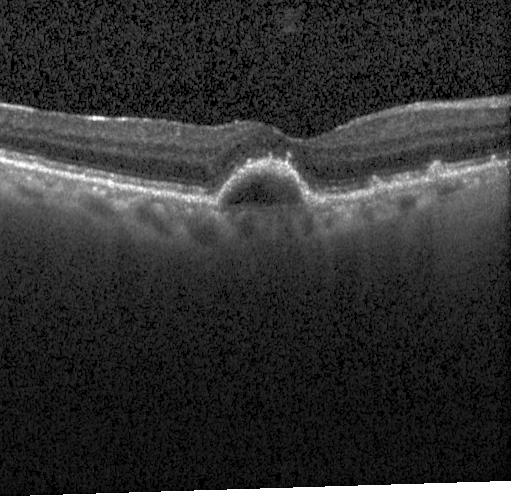 Choroidal neovascularization (CNV).